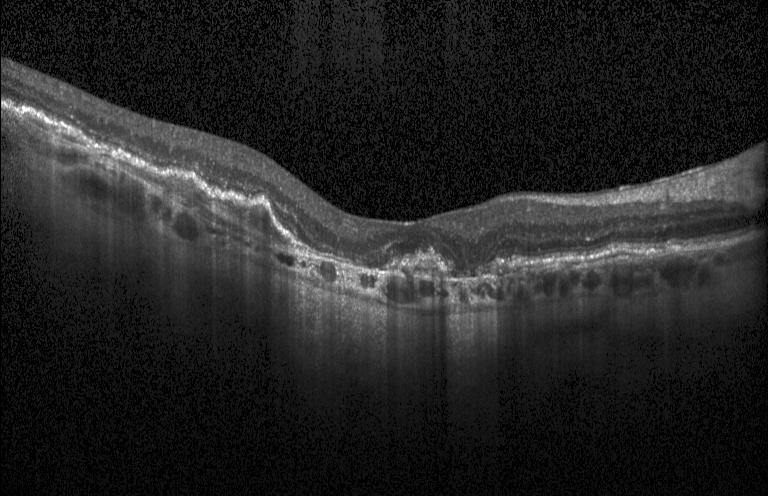

Optical coherence tomography B-scan, instrument: Heidelberg Spectralis, spectral-domain OCT, fovea-centered
Impression: choroidal neovascularization.